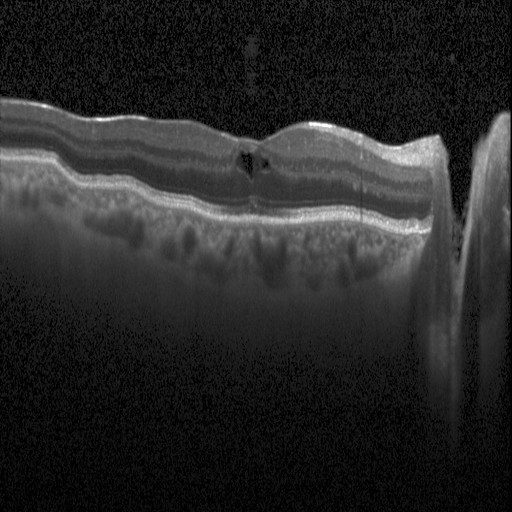
Acquired on a Heidelberg Spectralis, optical coherence tomography B-scan
Assessment: diabetic macular edema.